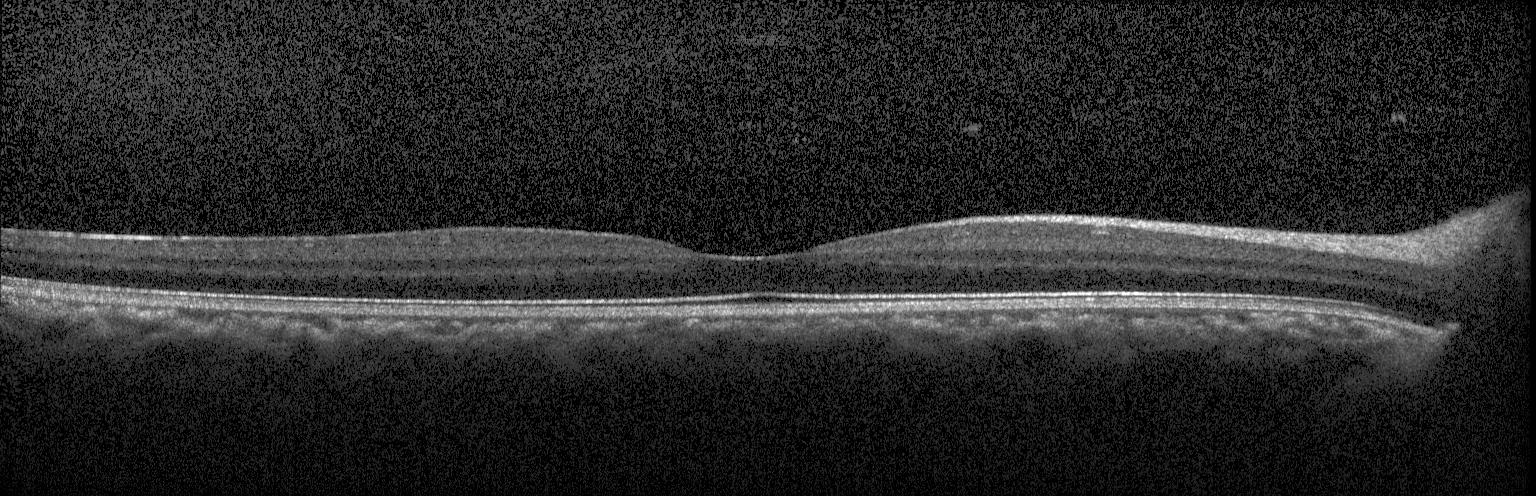 OCT B-scan, SD-OCT. Dx: no choroidal neovascularization, no diabetic macular edema, and no drusen.